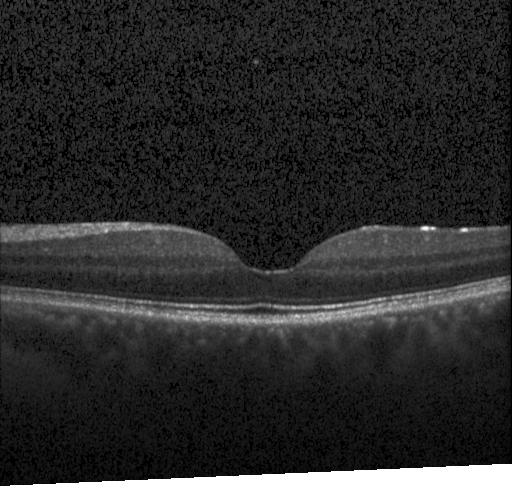 Retinal OCT B-scan. OCT finding: no evidence of choroidal neovascularization, diabetic macular edema, or drusen.